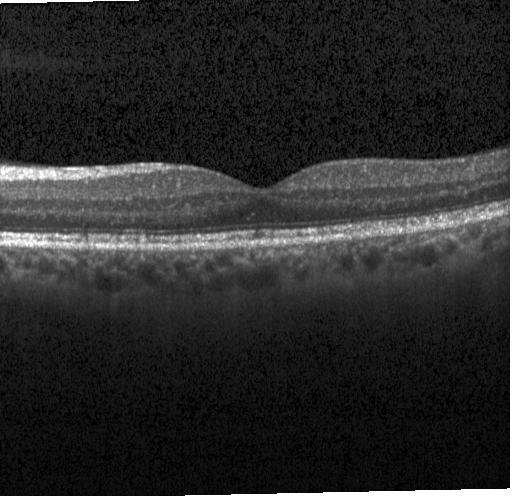 Spectral-domain OCT, OCT line scan, centered on the fovea, acquired on a Heidelberg Spectralis.
Finding: no choroidal neovascularization, diabetic macular edema, or drusen.